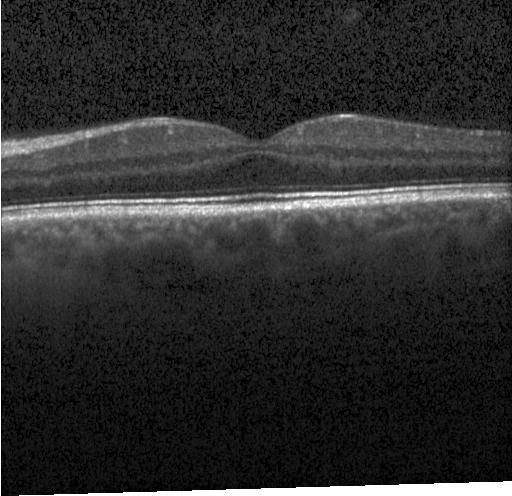 OCT line scan.
Diagnosis: no CNV, DME, or drusen.